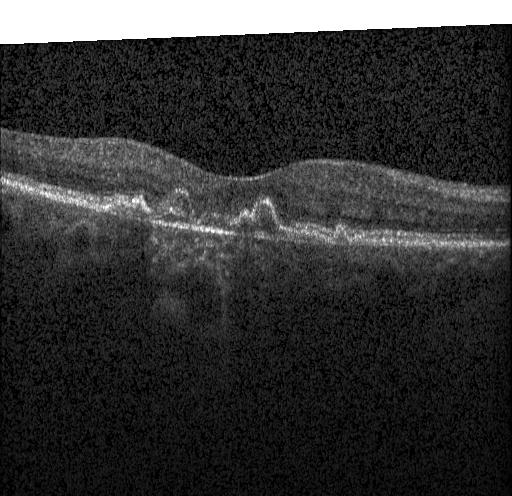

OCT finding: choroidal neovascularization (CNV).